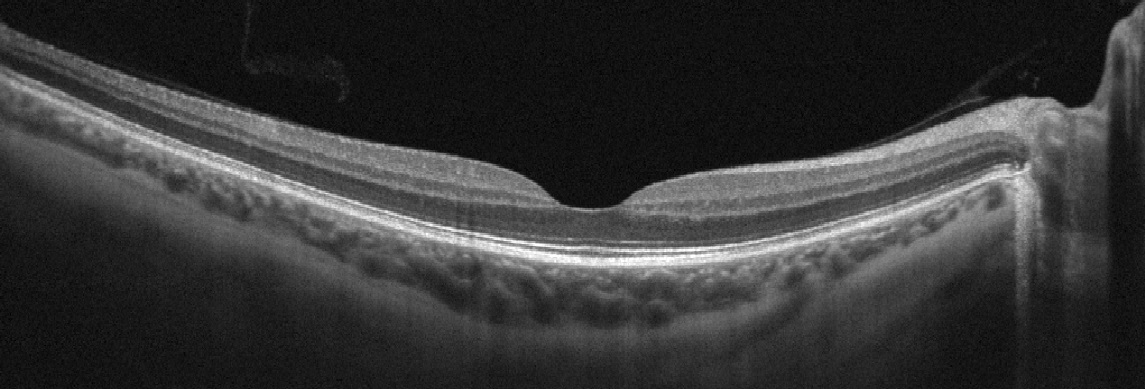
Diagnosis: no AMD, DME, ERM, RAO, RVO, or VID.